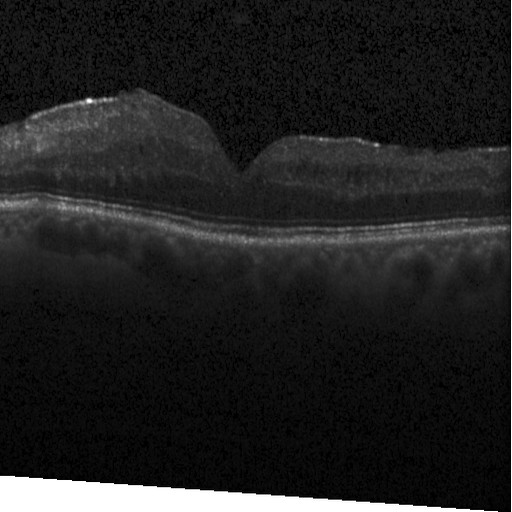

Horizontal scan through the fovea · retinal OCT B-scan · acquired on a Heidelberg Spectralis — Dx: DME.